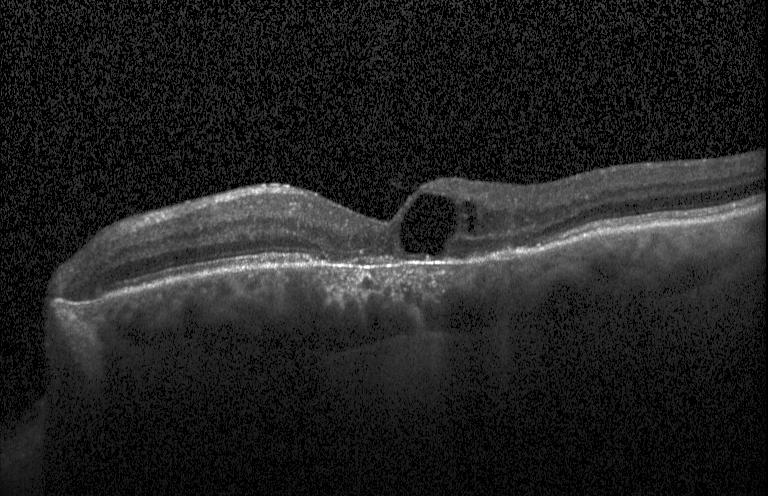
Finding: a choroidal neovascular membrane.